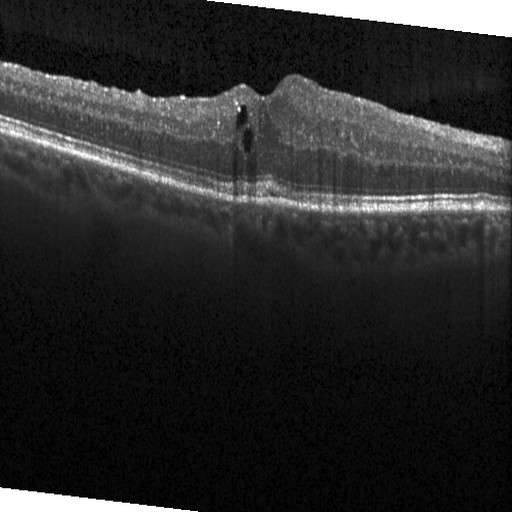 Diagnosis: diabetic macular edema.